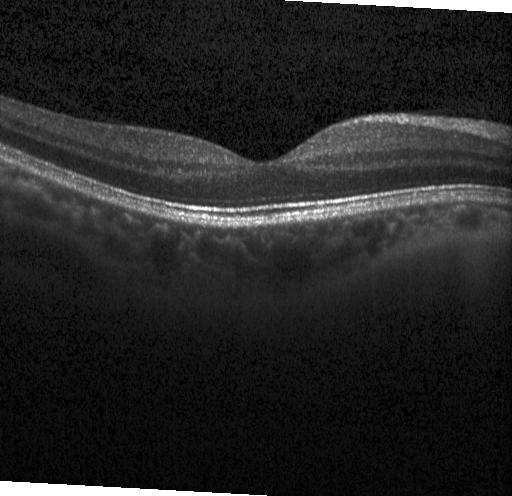

Heidelberg Spectralis. Through the macula. OCT line scan. Spectral-domain OCT
Dx: no choroidal neovascularization, diabetic macular edema, or drusen.